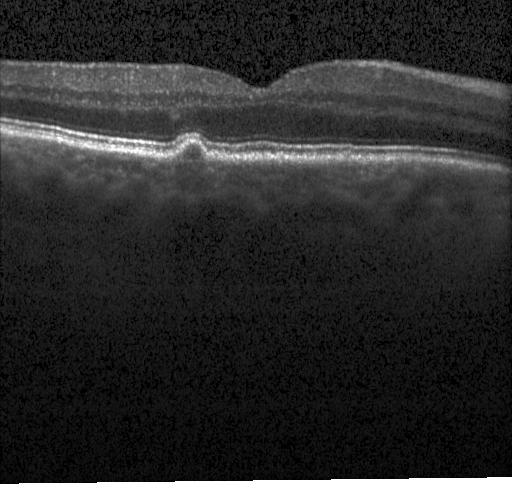
Spectral-domain optical coherence tomography · acquired on a Heidelberg Spectralis · retinal OCT cross-section.
Impression: multiple drusen.